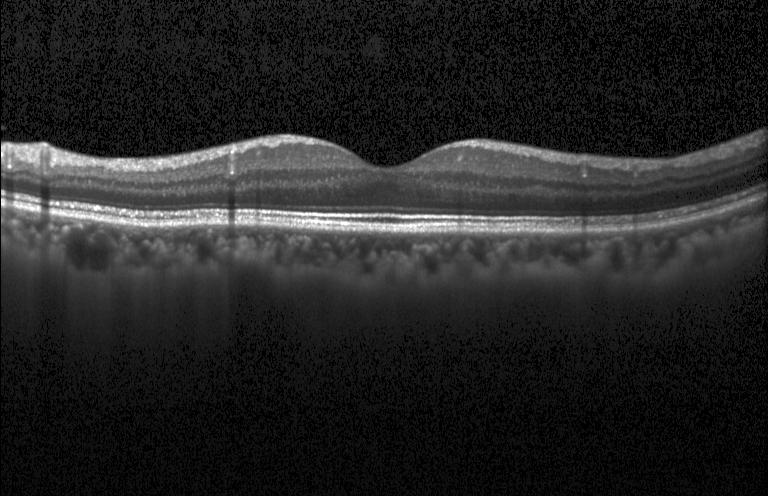
Spectral-domain OCT · centered on the fovea · Heidelberg Spectralis OCT system · optical coherence tomography B-scan.
This B-scan demonstrates no choroidal neovascularization, diabetic macular edema, or drusen.